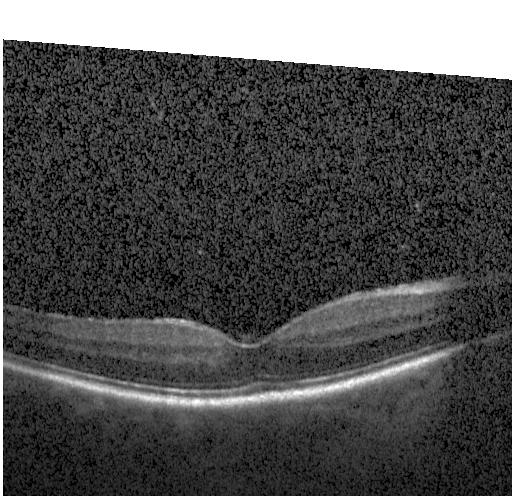
Macular OCT demonstrating no evidence of CNV, DME, or drusen.